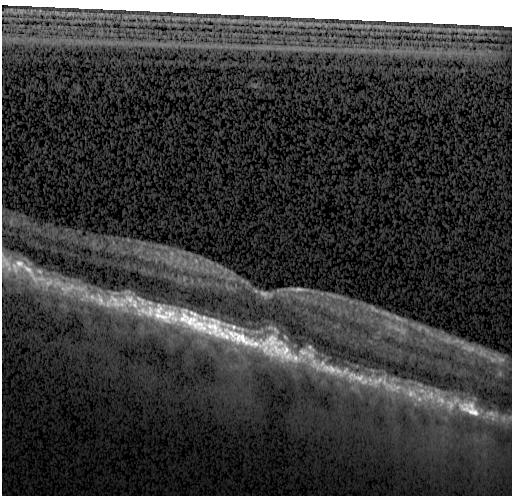

Optical coherence tomography scan · Heidelberg Spectralis. Finding: multiple drusen.